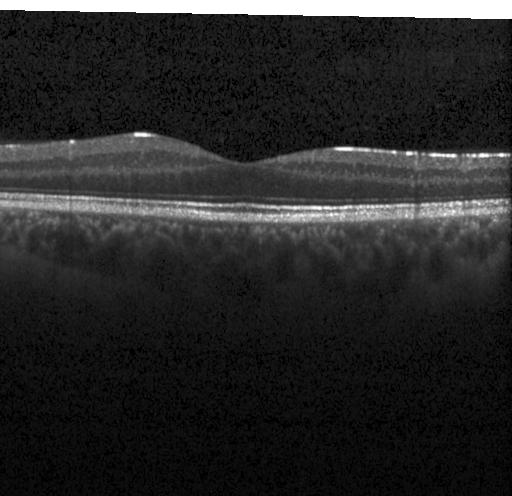
Spectral-domain OCT; OCT B-scan; horizontal scan through the fovea; Heidelberg Spectralis OCT system. Impression: no evidence of CNV, DME, or drusen.